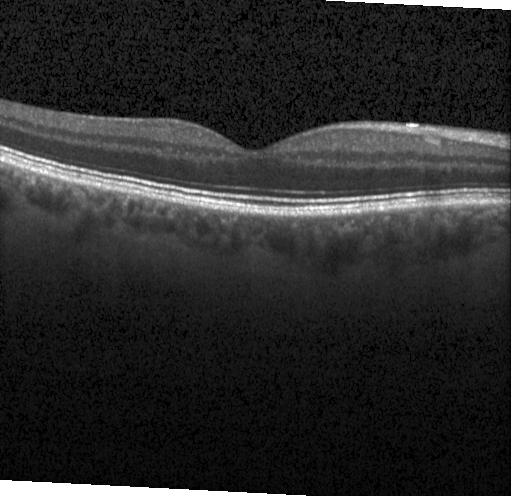
Macular OCT: no choroidal neovascularization, no diabetic macular edema, and no drusen.